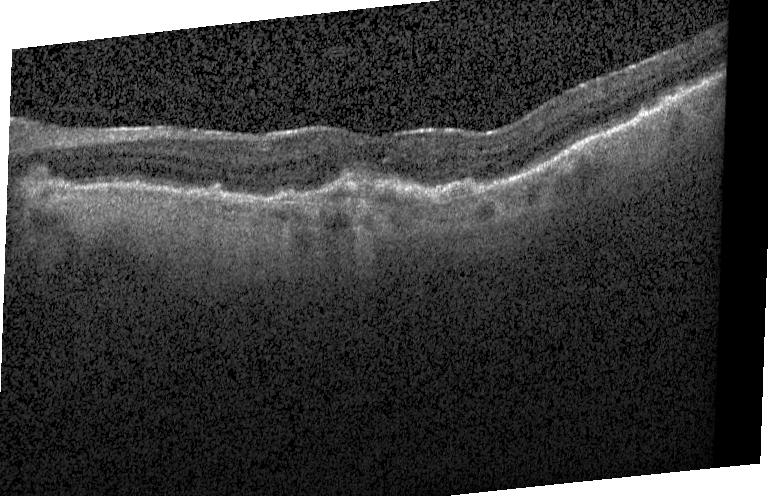 Retinal OCT cross-section; fovea-centered. Impression: a choroidal neovascular membrane.